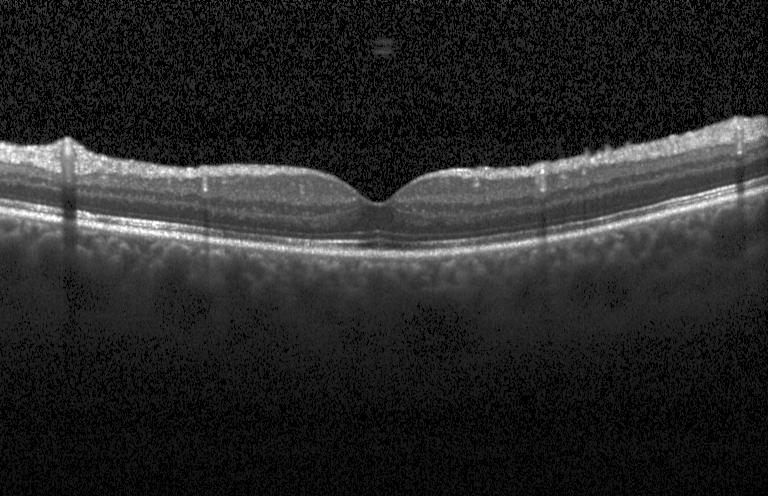 The scan shows no evidence of CNV, DME, or drusen.